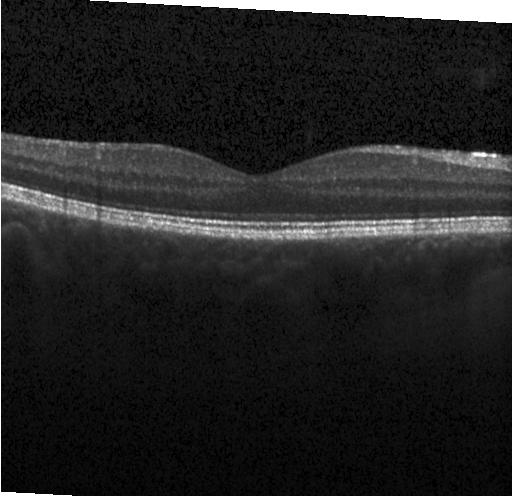
Diagnosis: no CNV, no DME, and no drusen.